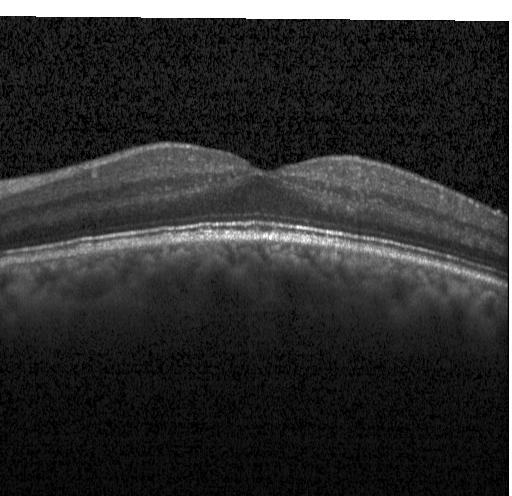 Retinal OCT cross-section showing no choroidal neovascularization, no diabetic macular edema, and no drusen.